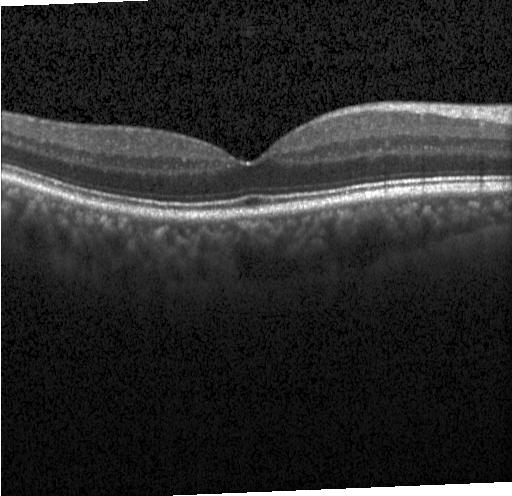
OCT line scan — Assessment: no choroidal neovascularization, diabetic macular edema, or drusen.